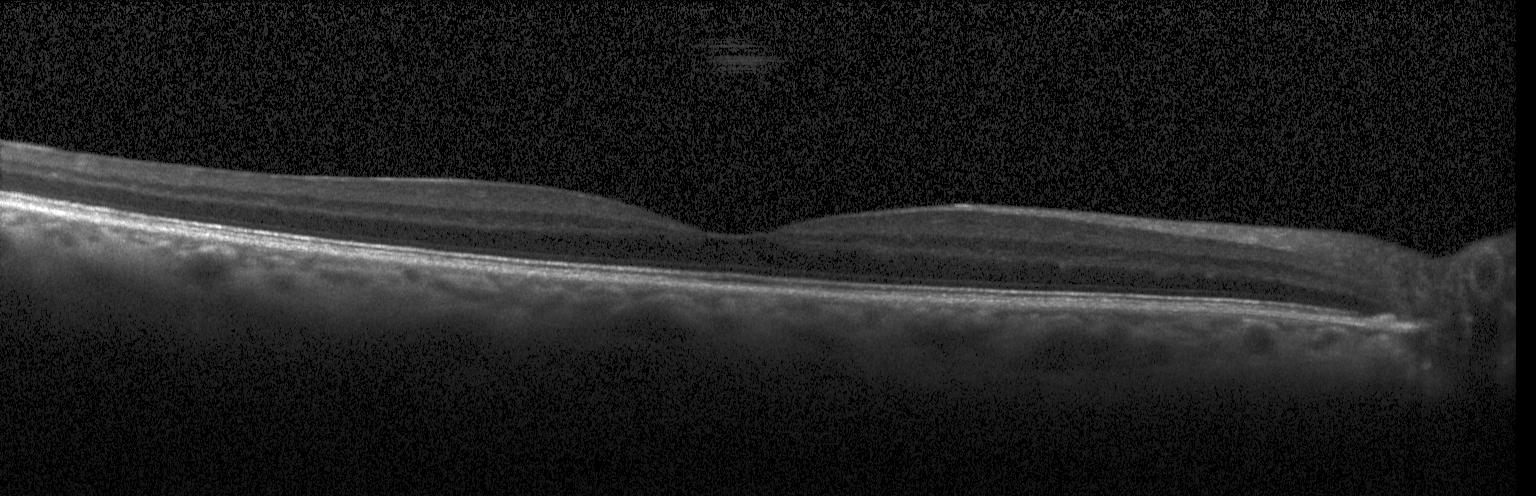

Optical coherence tomography B-scan
Diagnosis: neither CNV, DME, nor drusen.